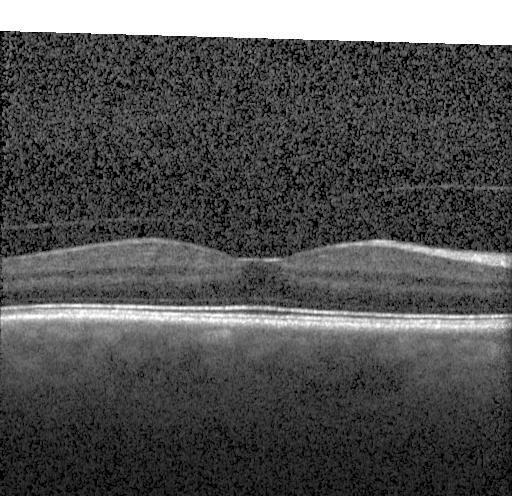 Dx: no choroidal neovascularization, diabetic macular edema, or drusen.